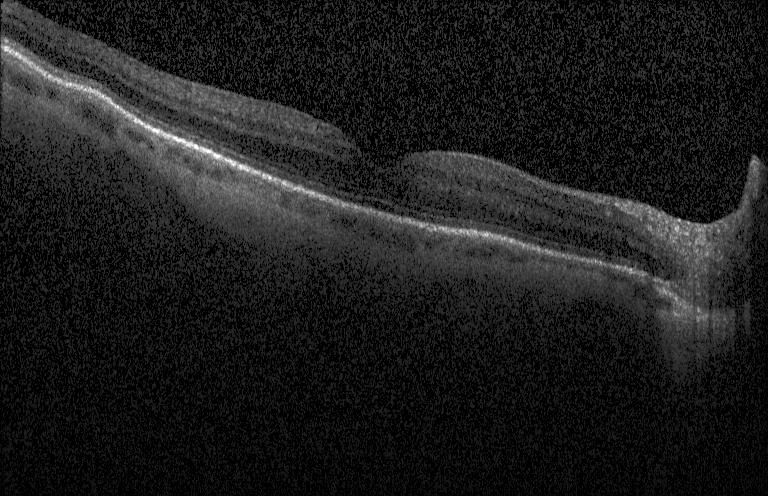 Retinal OCT B-scan. Diagnosis: no CNV, DME, or drusen.